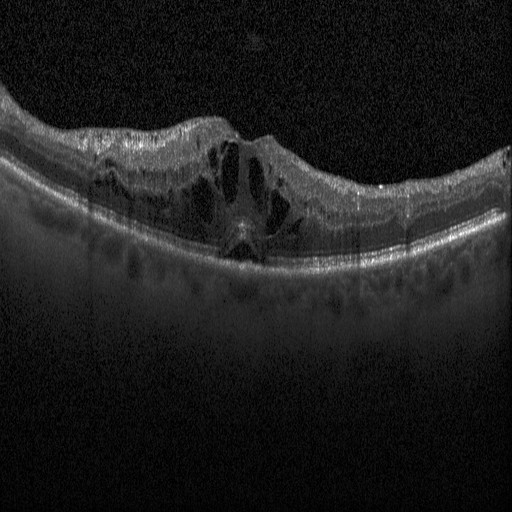
Heidelberg Spectralis OCT system, macular scan, OCT B-scan. Dx: diabetic macular edema (DME).